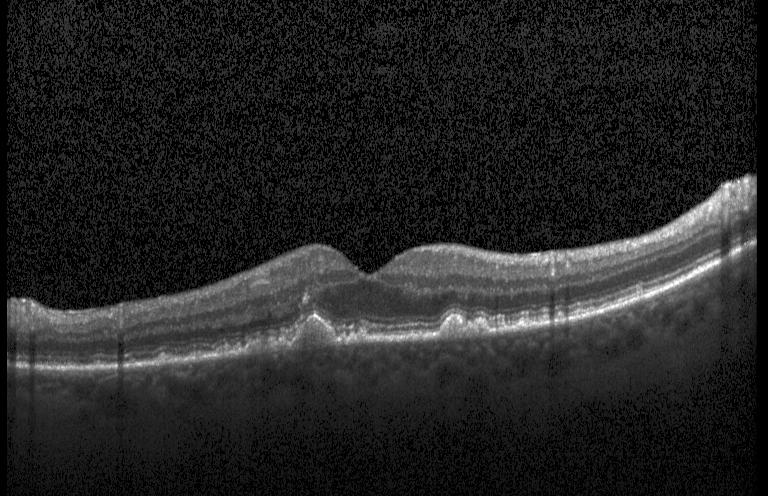

Diagnosis: drusen.